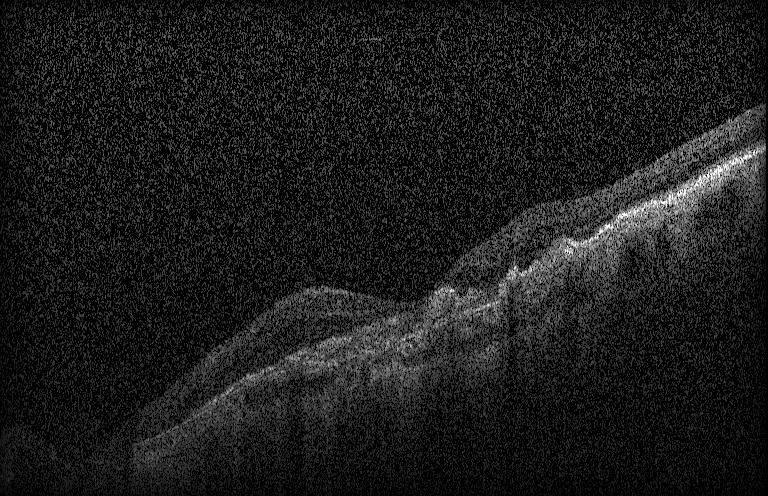 Retinal OCT B-scan.
Diagnosis: choroidal neovascularization.